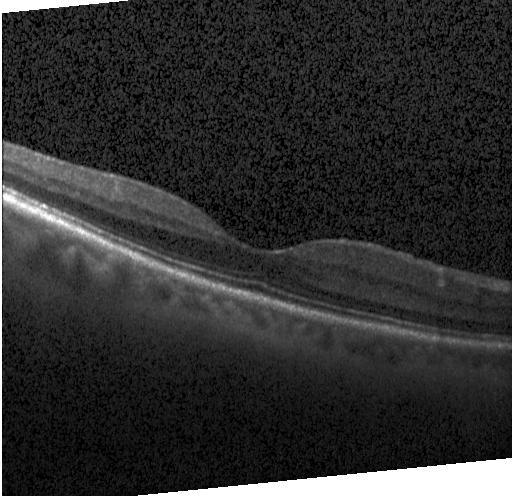 Diagnosis: no evidence of CNV, DME, or drusen.